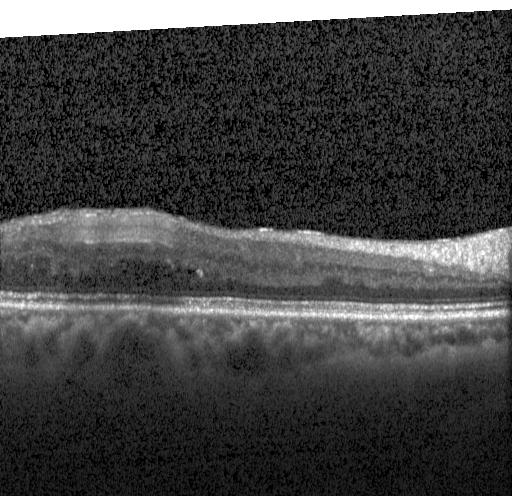 Spectral-domain optical coherence tomography; retinal OCT cross-section — This B-scan demonstrates DME.